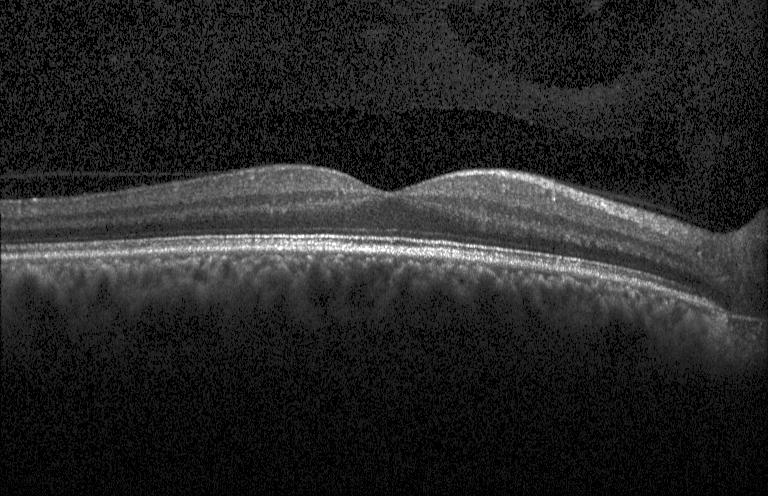 Heidelberg Spectralis, OCT line scan.
The scan shows no evidence of choroidal neovascularization, diabetic macular edema, or drusen.